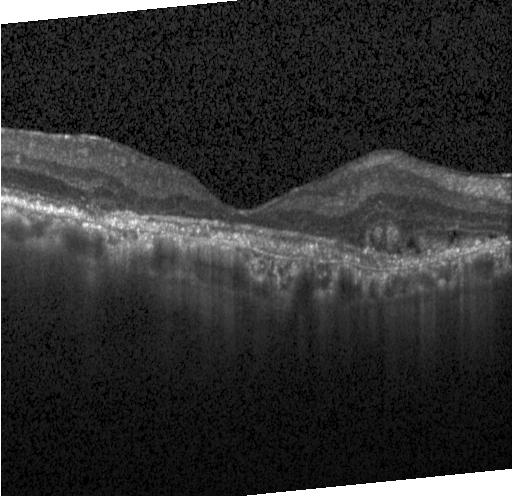

SD-OCT, optical coherence tomography scan, Heidelberg Spectralis OCT system. Finding: a choroidal neovascular membrane.